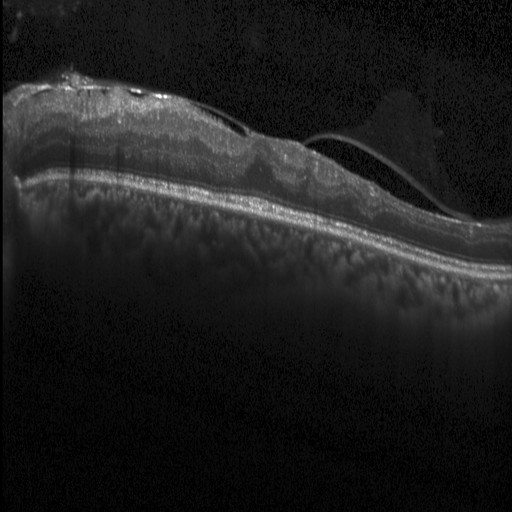

Retinal OCT cross-section showing diabetic macular edema (DME).